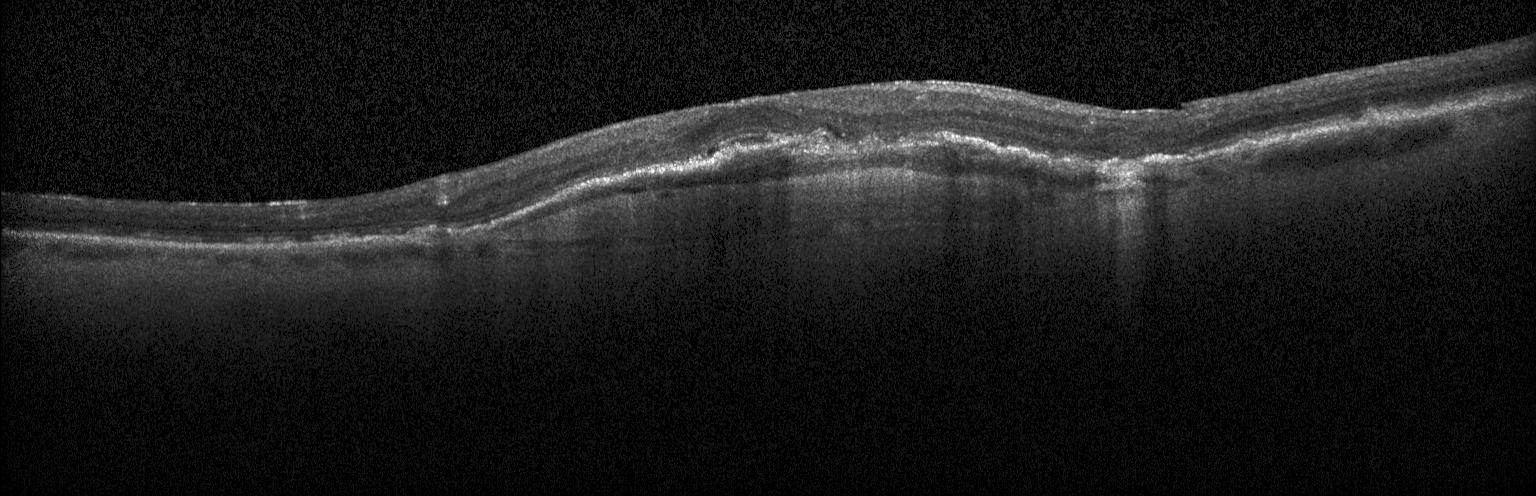

Retinal OCT cross-section showing a choroidal neovascular membrane.